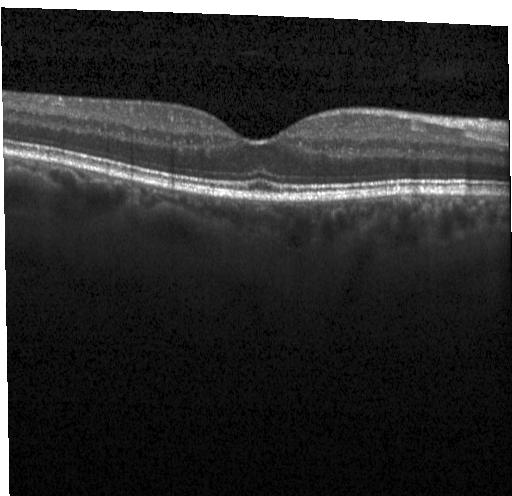
Spectral-domain OCT. Acquired on a Heidelberg Spectralis. Retinal OCT cross-section — Finding: no evidence of CNV, DME, or drusen.